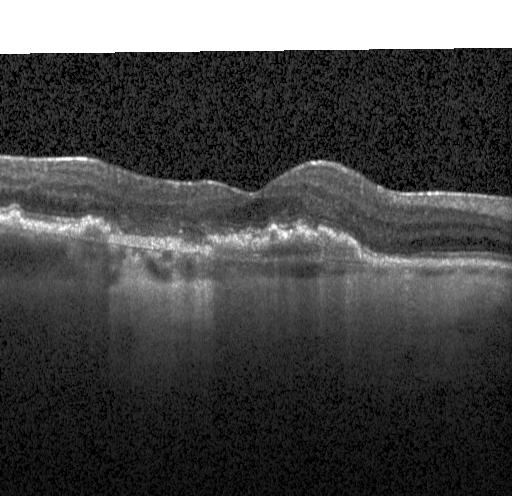

Dx: choroidal neovascularization.